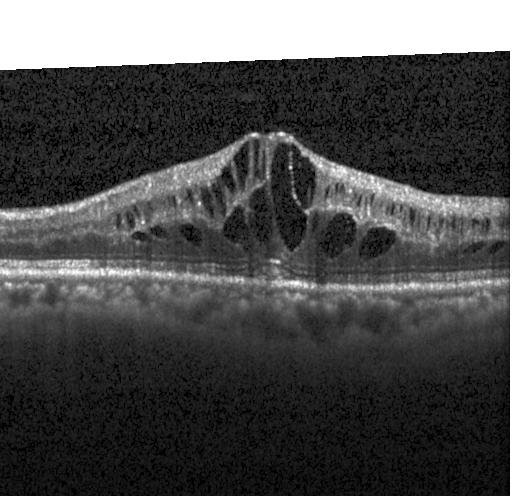
Retinal OCT B-scan
Finding: diabetic macular edema (DME).